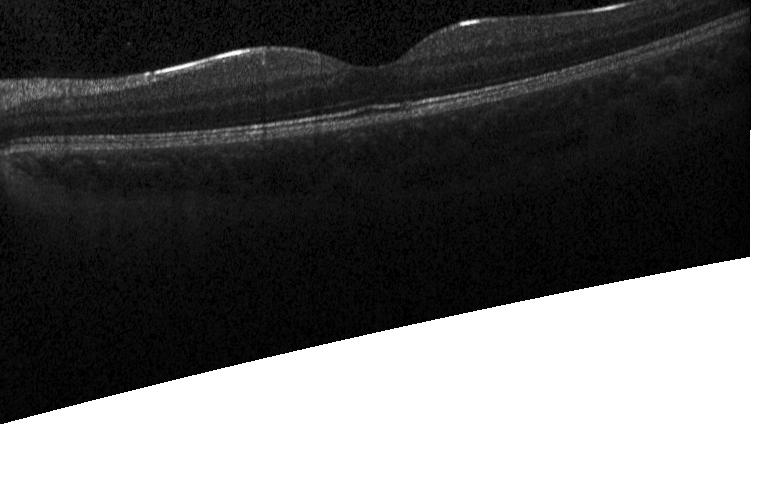
OCT line scan — Impression: no choroidal neovascularization, no diabetic macular edema, and no drusen.